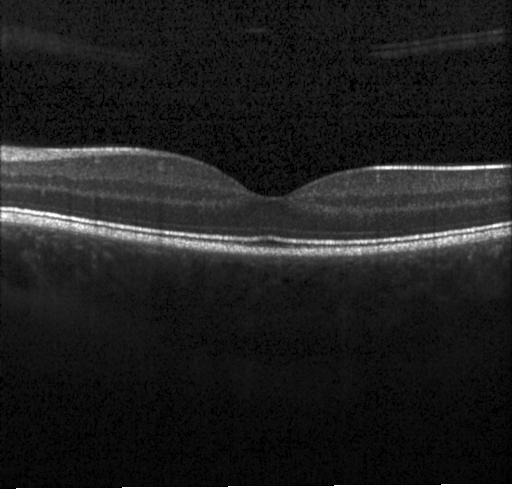

Heidelberg Spectralis OCT system. SD-OCT. Centered on the fovea. Retinal OCT cross-section. Finding: neither choroidal neovascularization, diabetic macular edema, nor drusen.